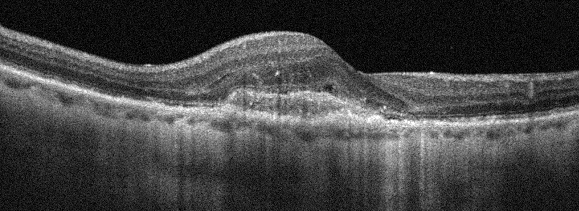
OD, optical coherence tomography B-scan. Finding: age-related macular degeneration (AMD).